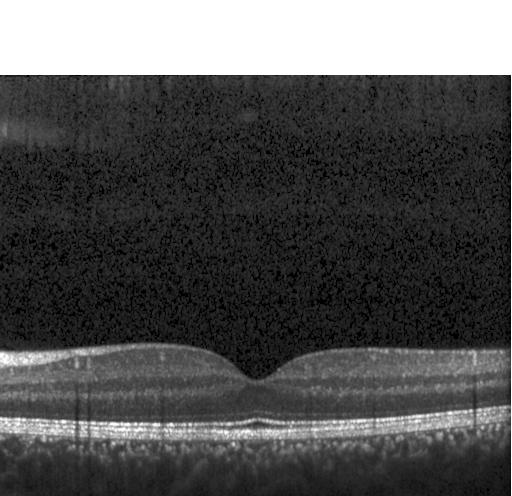
The scan shows neither choroidal neovascularization, diabetic macular edema, nor drusen.